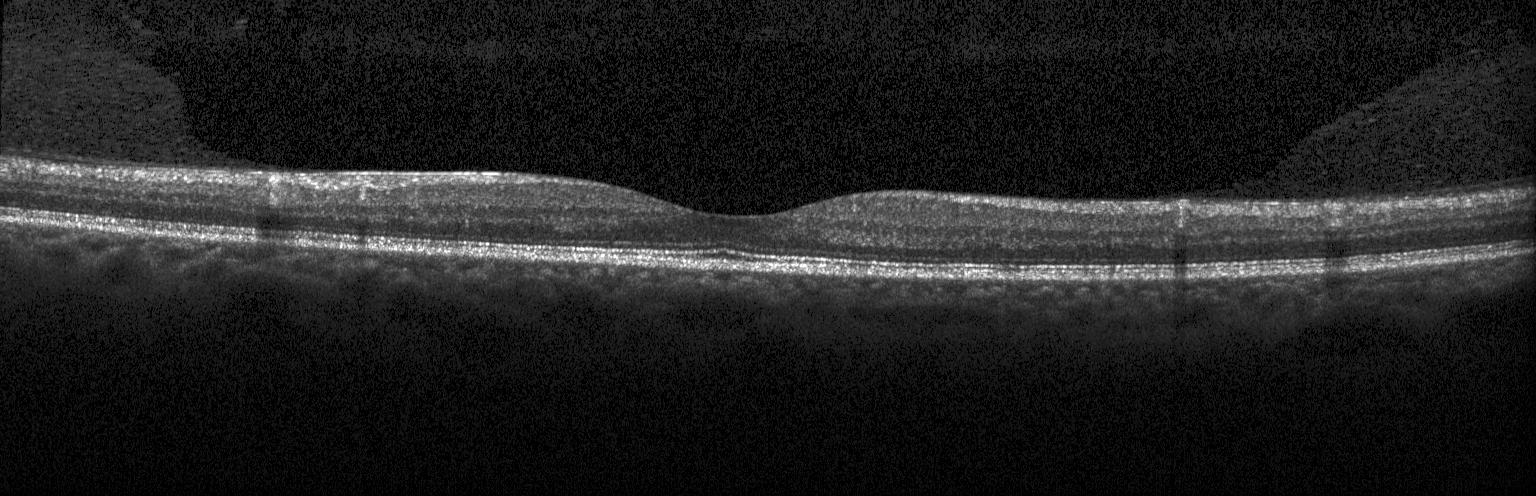

Retinal OCT cross-section; through the macula
Impression: no evidence of CNV, DME, or drusen.